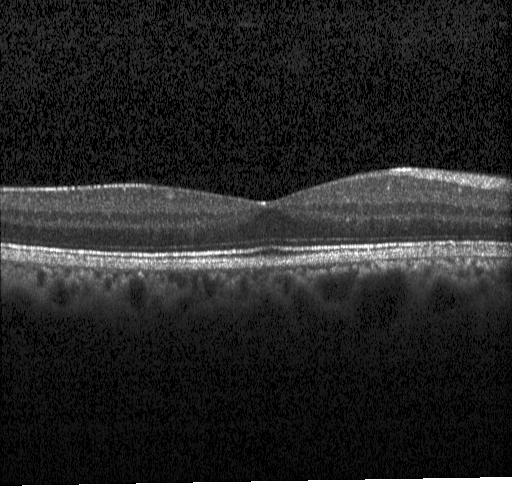 Dx: no CNV, no DME, and no drusen.